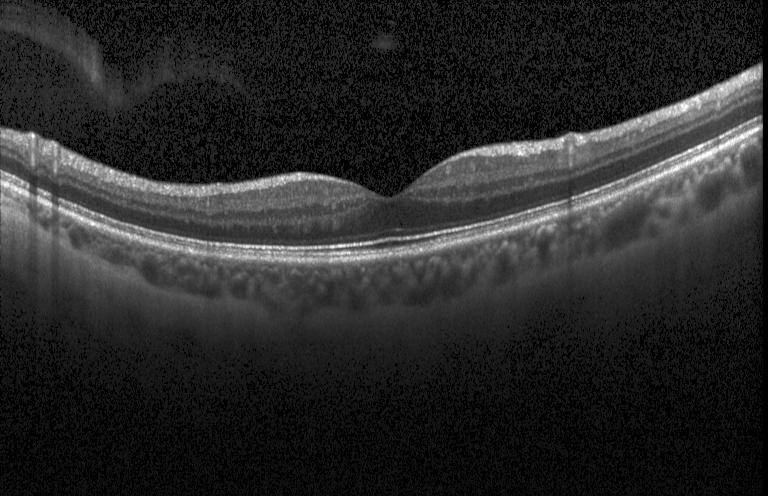

Fovea-centered · retinal OCT B-scan
Neither choroidal neovascularization, diabetic macular edema, nor drusen.